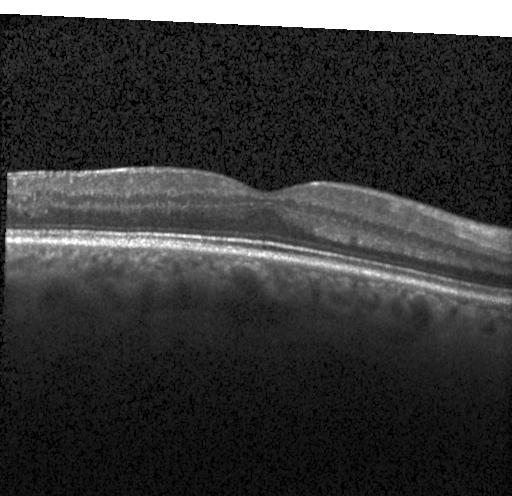

Spectral-domain OCT; centered on the fovea; retinal OCT B-scan; Heidelberg Spectralis OCT system. Diagnosis: no evidence of choroidal neovascularization, diabetic macular edema, or drusen.